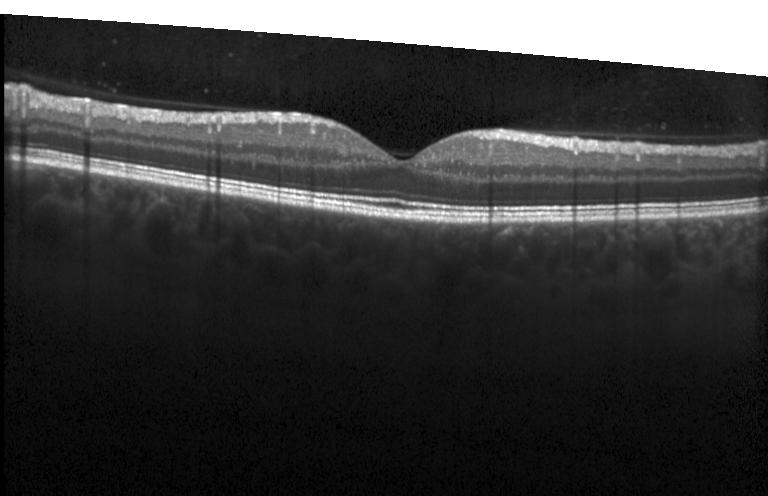
Retinal OCT cross-section · horizontal scan through the fovea.
Finding: neither choroidal neovascularization, diabetic macular edema, nor drusen.